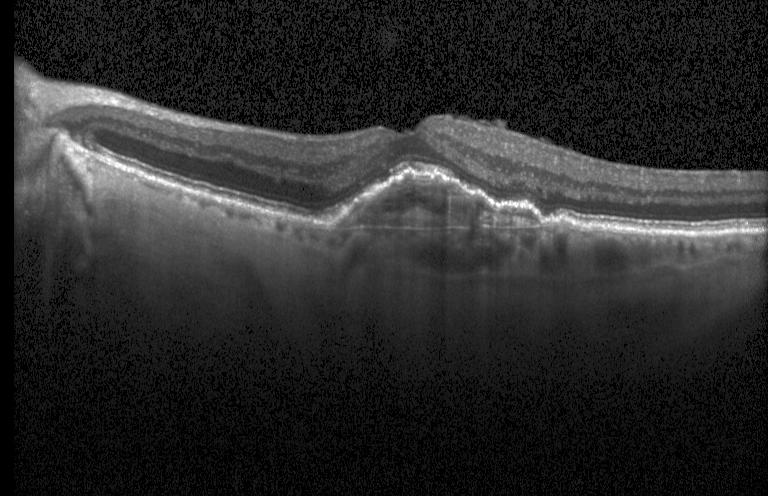
SD-OCT, instrument: Heidelberg Spectralis, centered on the fovea, OCT line scan
This B-scan demonstrates choroidal neovascularization (CNV).